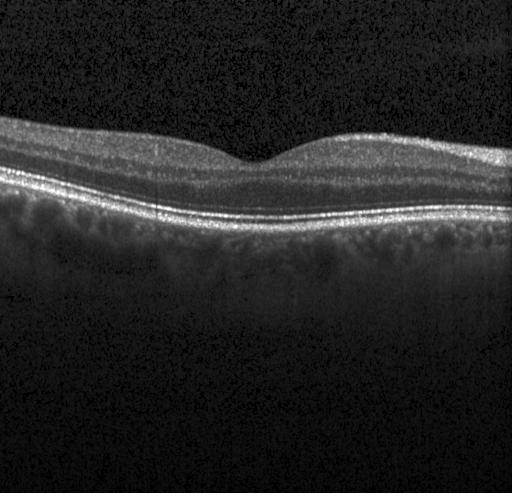 Impression: no evidence of CNV, DME, or drusen.